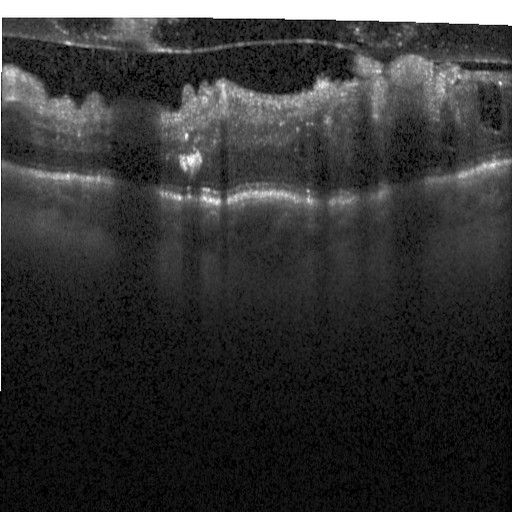
OCT scan showing DME.